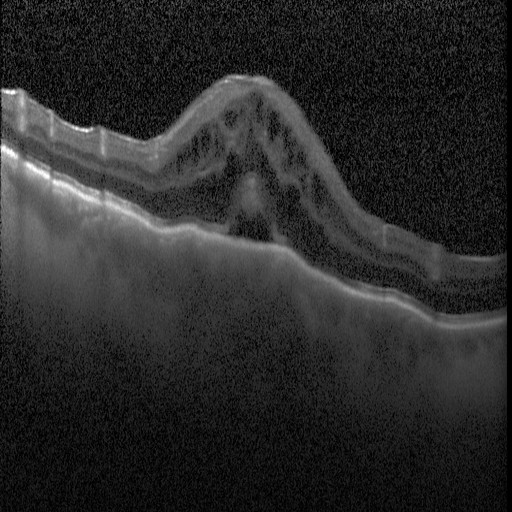

Diagnosis: diabetic macular edema (DME).